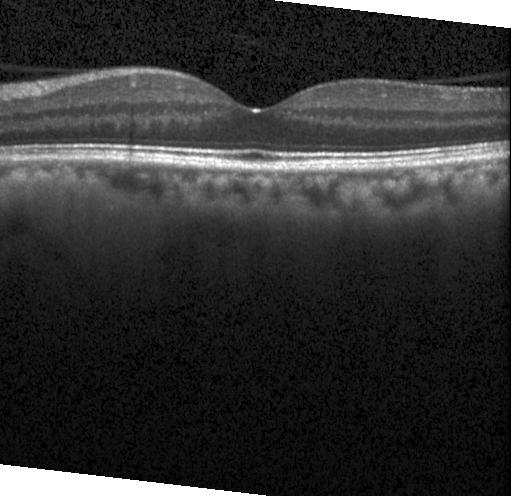

Macular OCT: neither choroidal neovascularization, diabetic macular edema, nor drusen.